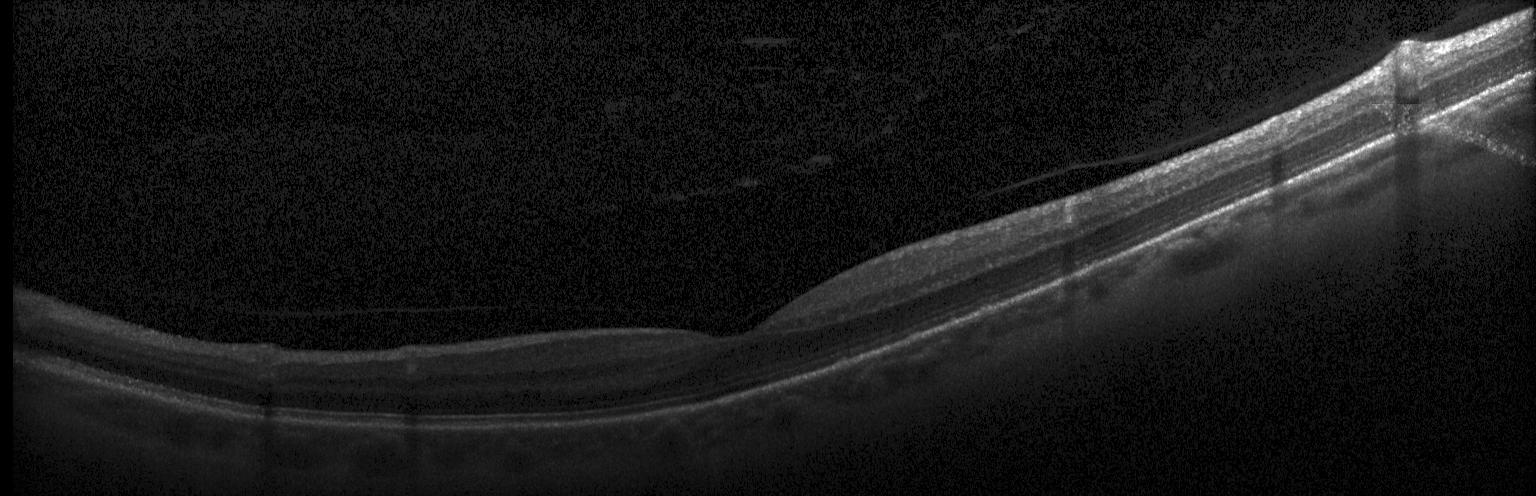
Diagnosis: no evidence of CNV, DME, or drusen.